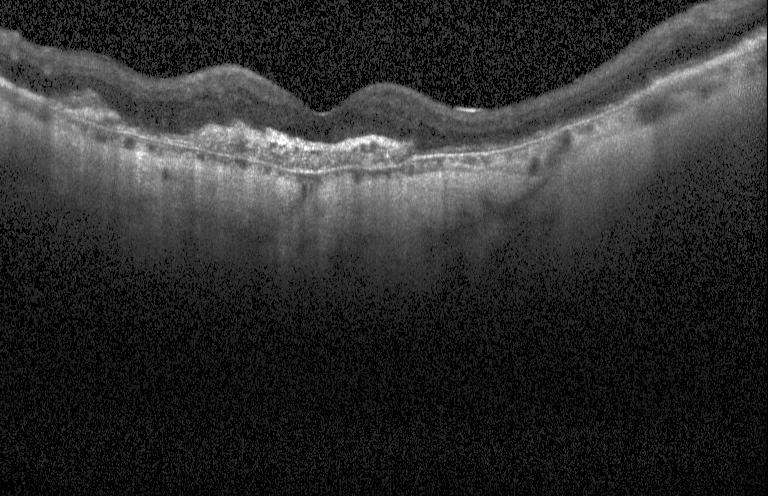

The scan shows a choroidal neovascular membrane.